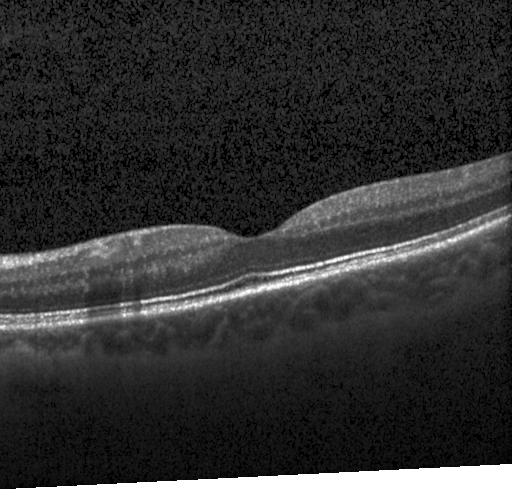 Optical coherence tomography B-scan. Acquired on a Heidelberg Spectralis
Finding: no evidence of choroidal neovascularization, diabetic macular edema, or drusen.